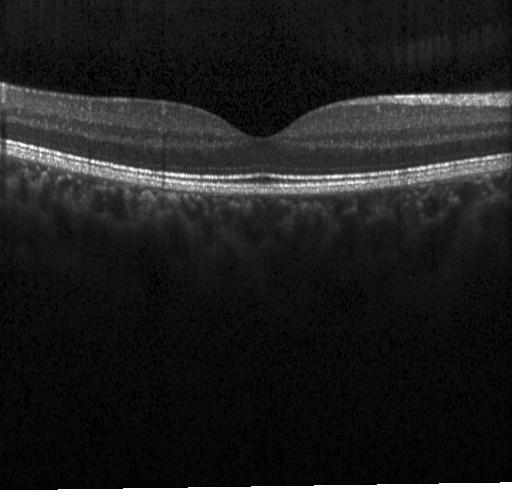 Macular OCT demonstrating neither choroidal neovascularization, diabetic macular edema, nor drusen.